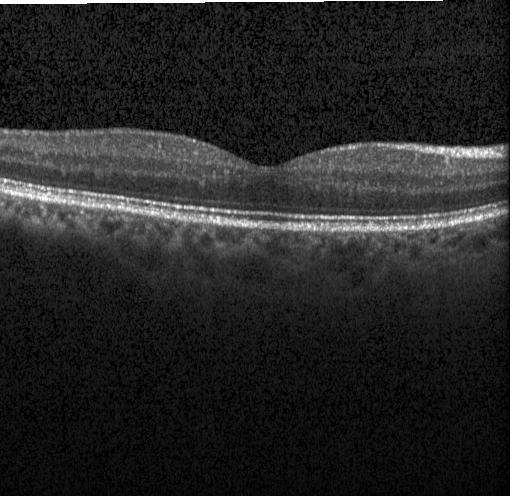

OCT scan showing neither CNV, DME, nor drusen.